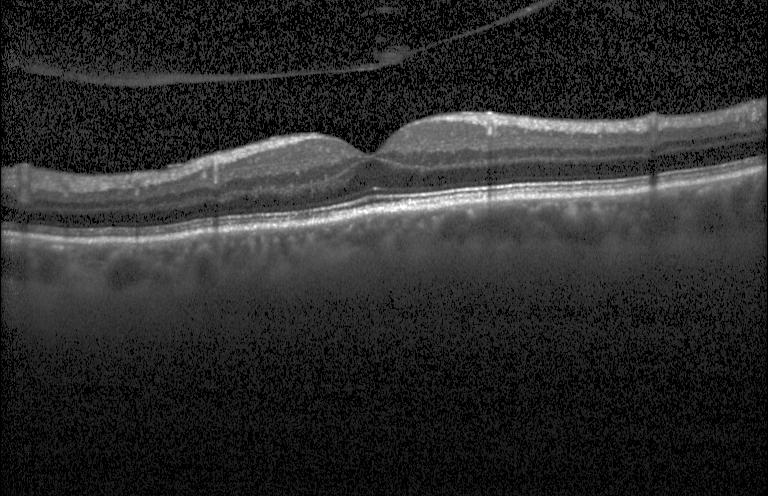 OCT B-scan
Impression: no CNV, no DME, and no drusen.